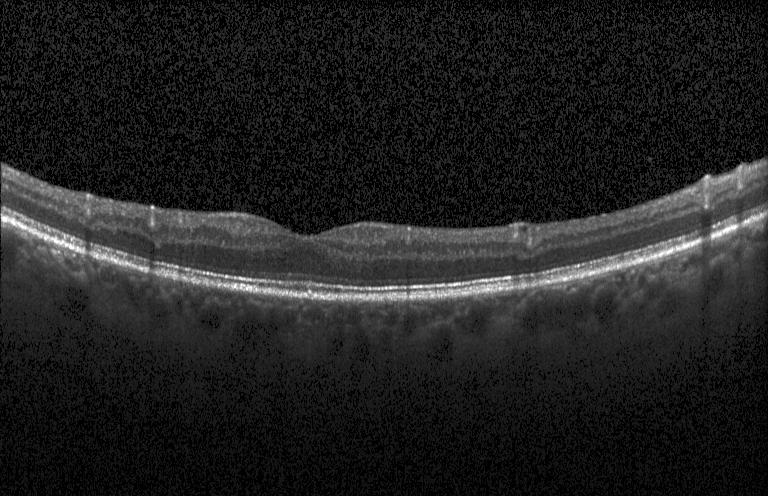 Retinal OCT B-scan. Instrument: Heidelberg Spectralis — Finding: no evidence of CNV, DME, or drusen.